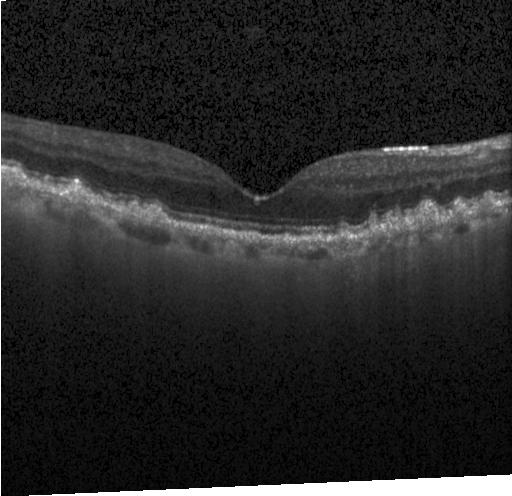
Impression: sub-RPE drusenoid deposits.